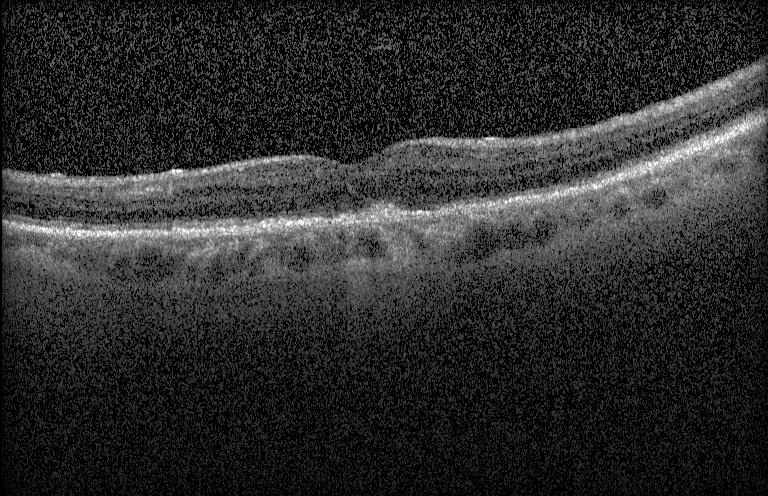 Spectral-domain OCT B-scan: a choroidal neovascular membrane.